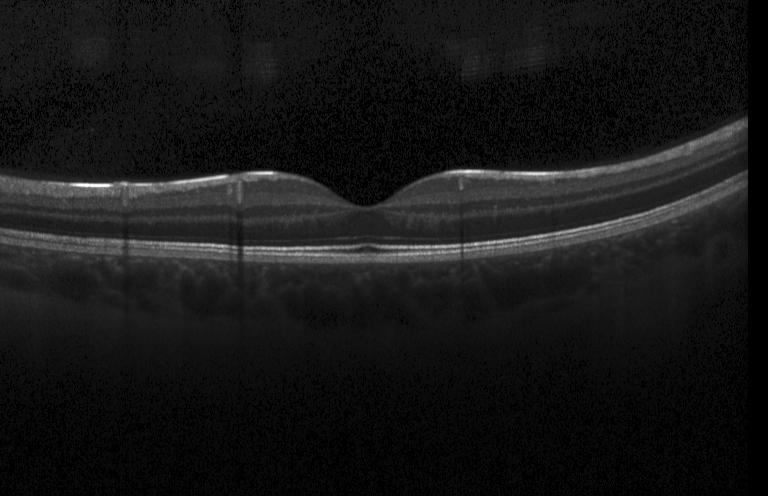
Heidelberg Spectralis OCT system; OCT line scan; centered on the fovea; spectral-domain OCT — Macular OCT: no choroidal neovascularization, diabetic macular edema, or drusen.